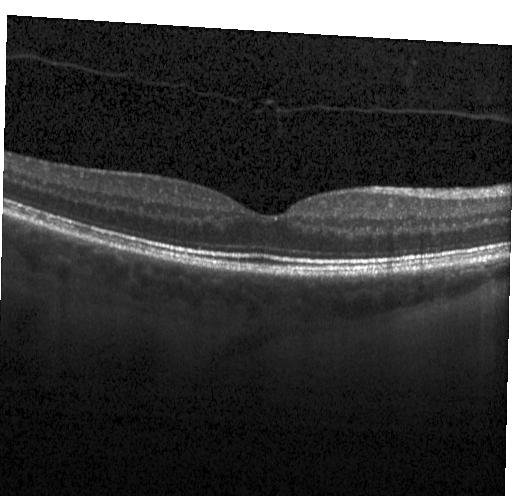

OCT B-scan, spectral-domain optical coherence tomography
Neither CNV, DME, nor drusen.